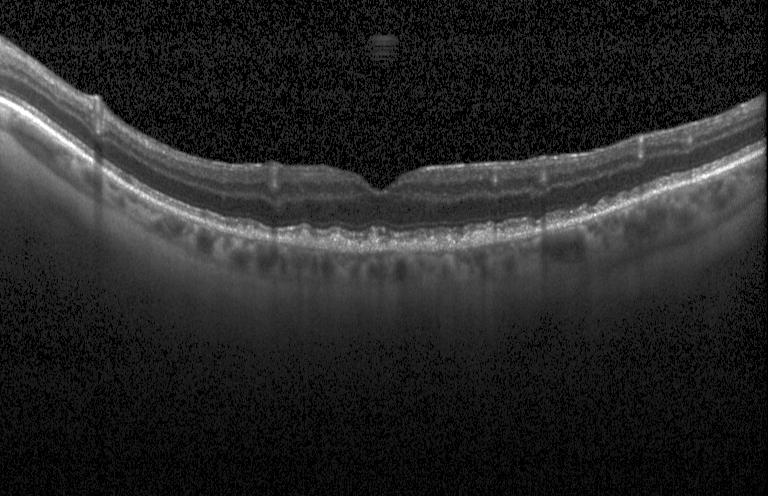

Centered on the fovea. Instrument: Heidelberg Spectralis. Retinal OCT B-scan — This B-scan demonstrates multiple drusen.